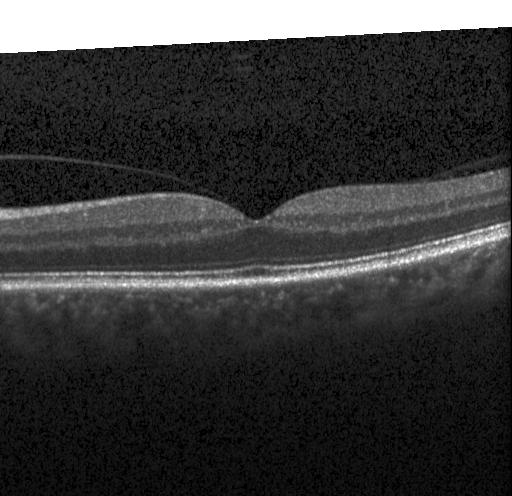
Impression: no CNV, DME, or drusen.